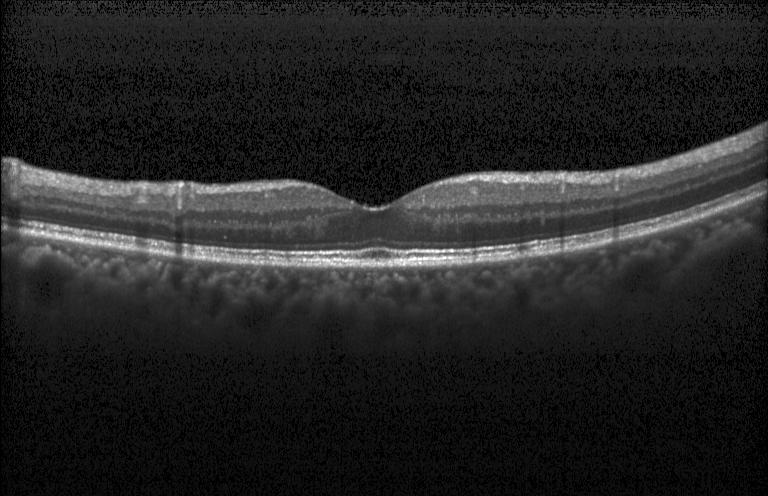
OCT finding: no evidence of choroidal neovascularization, diabetic macular edema, or drusen.